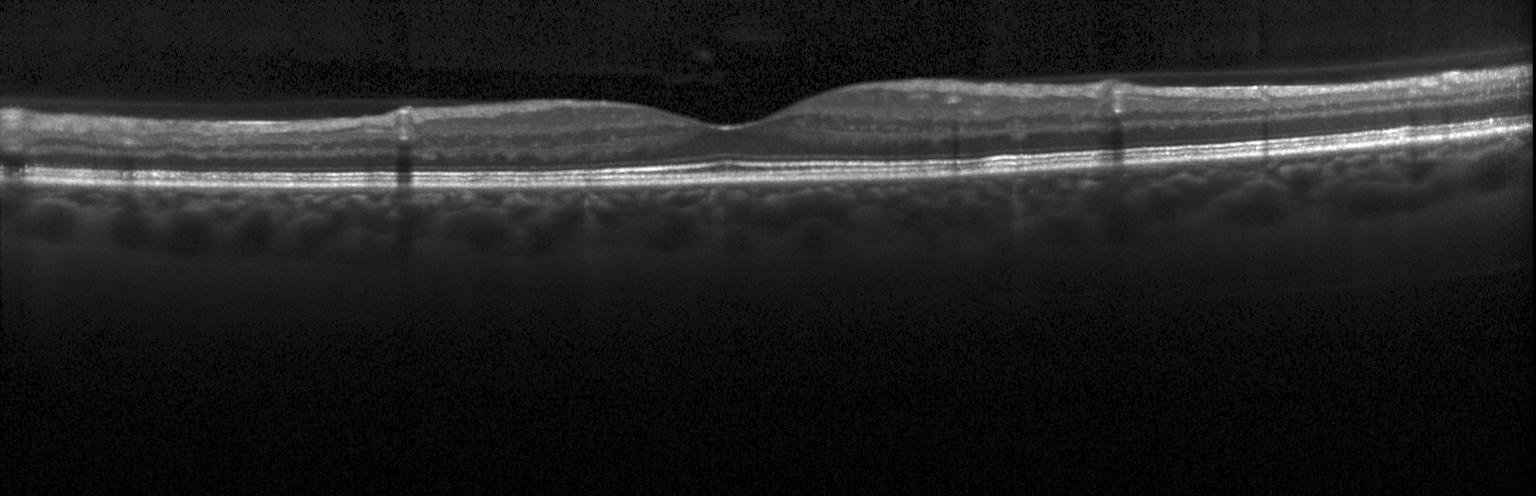 Assessment: no choroidal neovascularization, diabetic macular edema, or drusen.